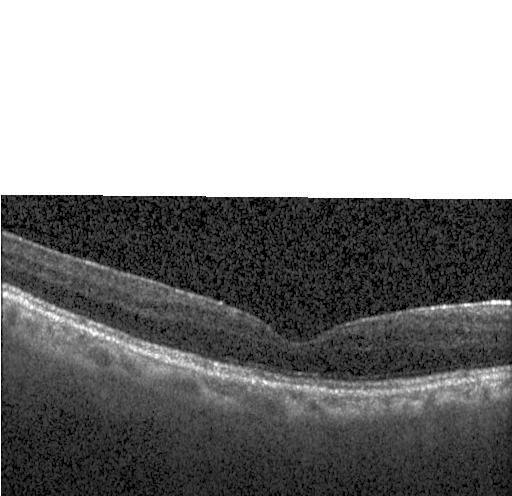 Heidelberg Spectralis OCT system, centered on the fovea, SD-OCT, OCT line scan.
Macular OCT: no CNV, DME, or drusen.